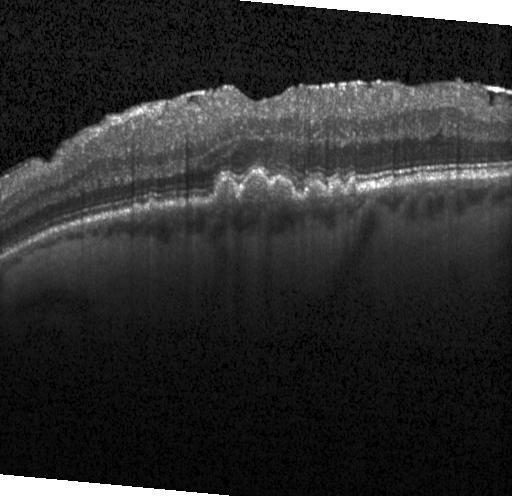 Spectral-domain OCT; Heidelberg Spectralis; horizontal scan through the fovea; retinal OCT B-scan
The scan shows drusen.